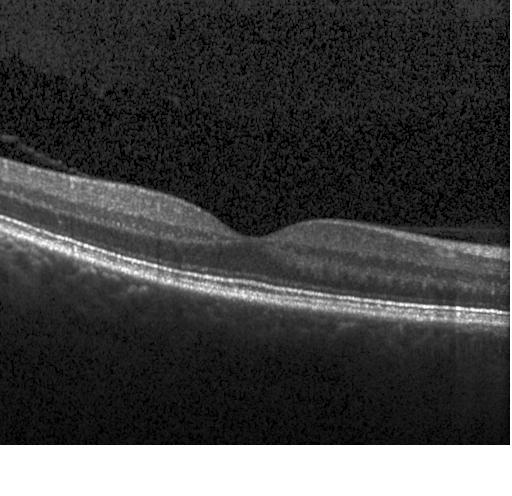
Macular scan, optical coherence tomography scan.
Diagnosis: no evidence of CNV, DME, or drusen.